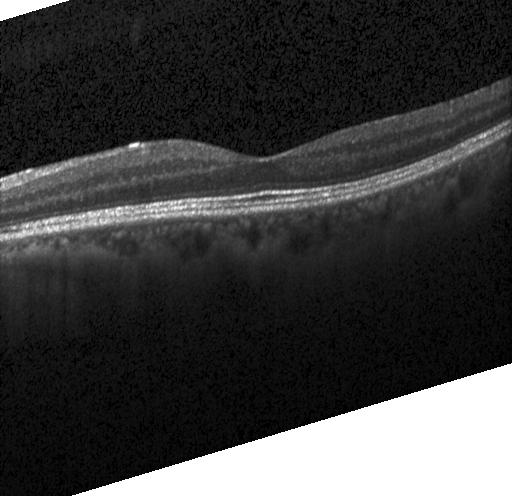 OCT finding: no choroidal neovascularization, diabetic macular edema, or drusen.